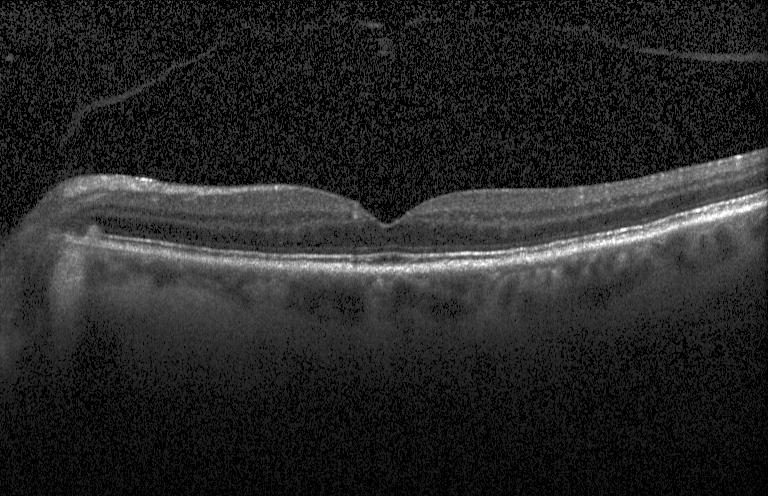
Finding: neither choroidal neovascularization, diabetic macular edema, nor drusen.